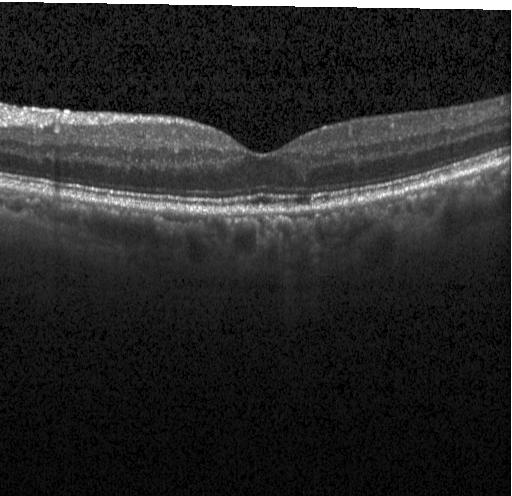 Finding: no CNV, no DME, and no drusen.